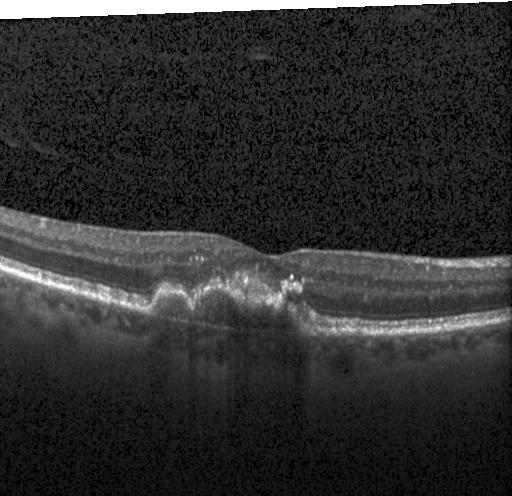

OCT line scan. Finding: choroidal neovascularization (CNV).